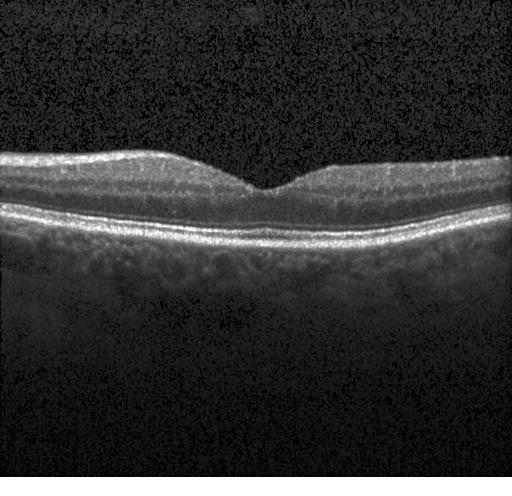
Macular OCT demonstrating no evidence of choroidal neovascularization, diabetic macular edema, or drusen.